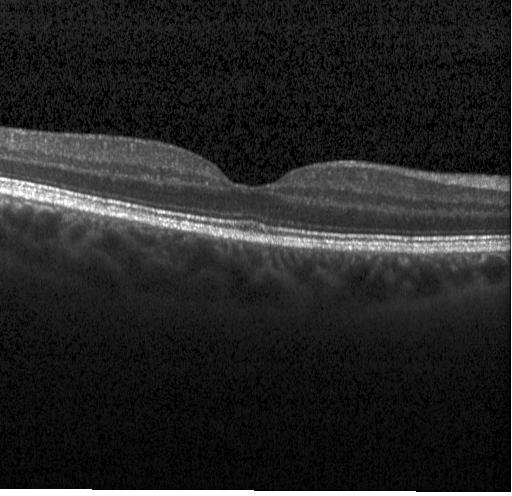

Centered on the fovea, retinal OCT B-scan, acquired on a Heidelberg Spectralis, spectral-domain optical coherence tomography
This B-scan demonstrates no CNV, DME, or drusen.